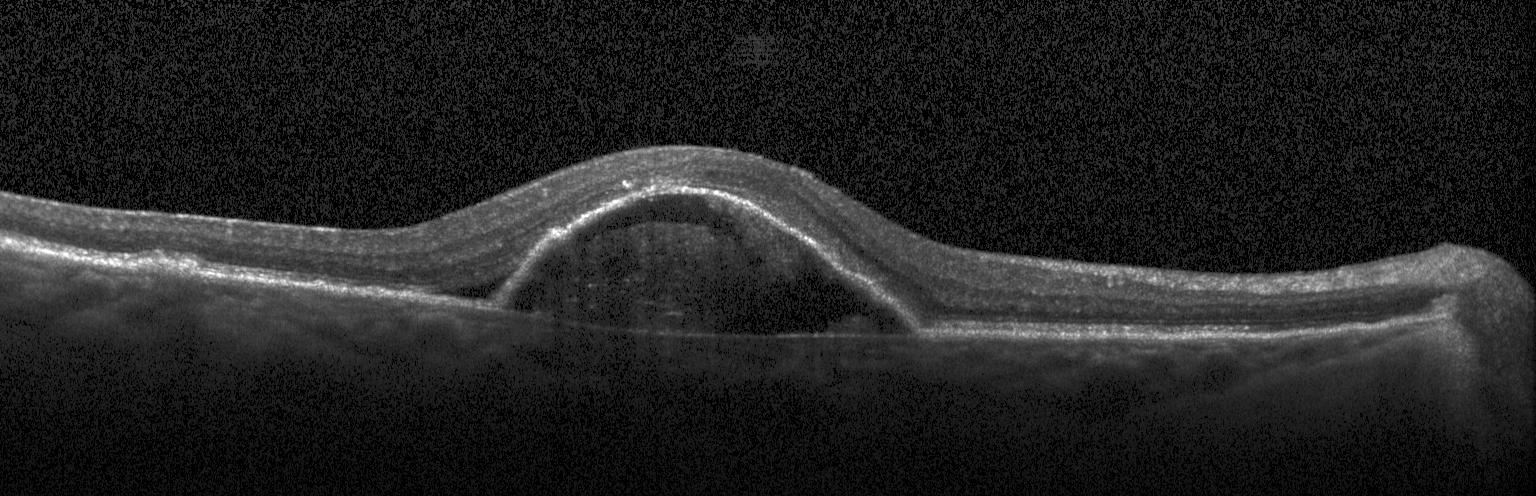 Spectral-domain OCT. OCT B-scan. Instrument: Heidelberg Spectralis.
OCT finding: CNV.